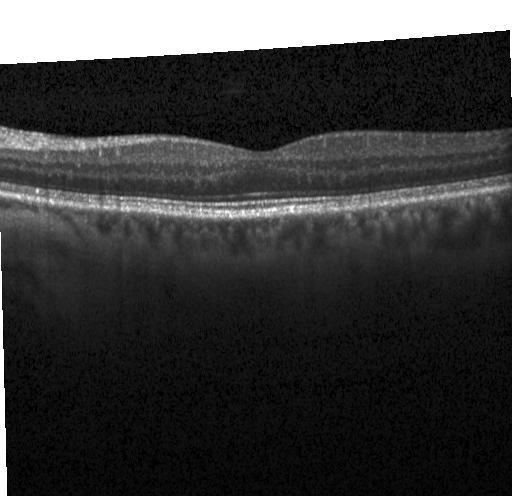

OCT B-scan showing no choroidal neovascularization, no diabetic macular edema, and no drusen.